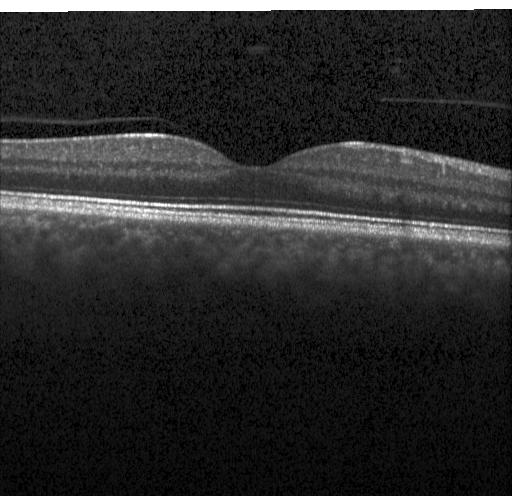 Macular OCT demonstrating no choroidal neovascularization, diabetic macular edema, or drusen.